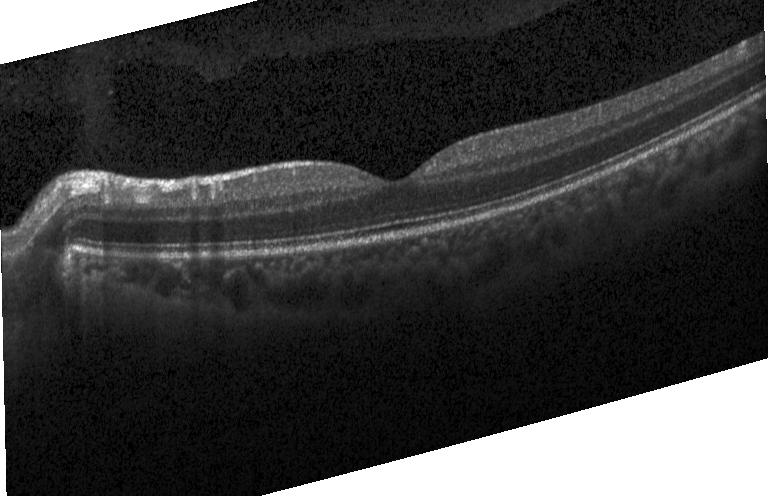
OCT line scan.
Diagnosis: neither choroidal neovascularization, diabetic macular edema, nor drusen.